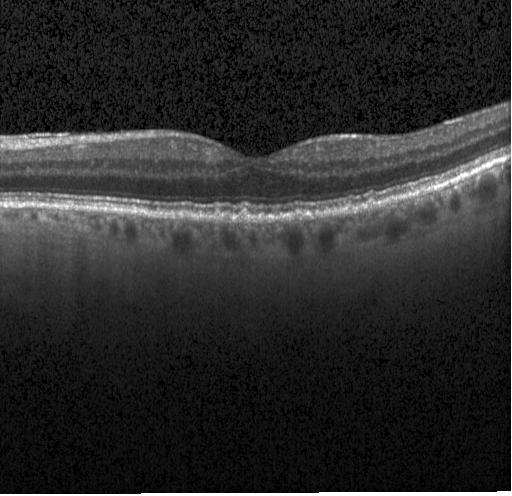
Through the macula; instrument: Heidelberg Spectralis; retinal OCT cross-section; spectral-domain optical coherence tomography.
Macular OCT: drusen.